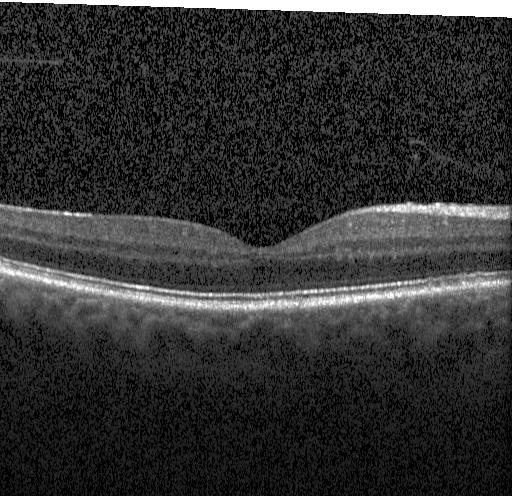 Heidelberg Spectralis OCT system. OCT line scan. Fovea-centered. SD-OCT.
Finding: no choroidal neovascularization, no diabetic macular edema, and no drusen.